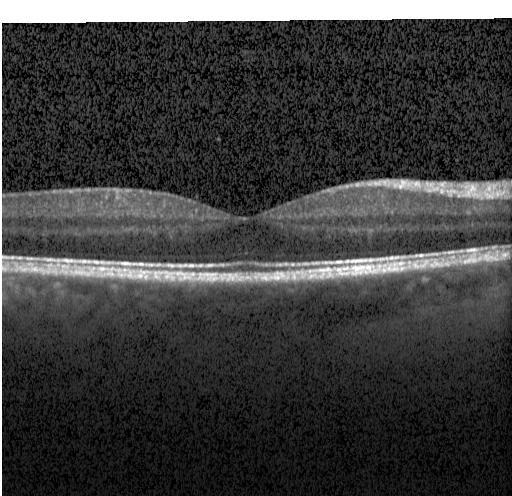 Diagnosis: no evidence of CNV, DME, or drusen.